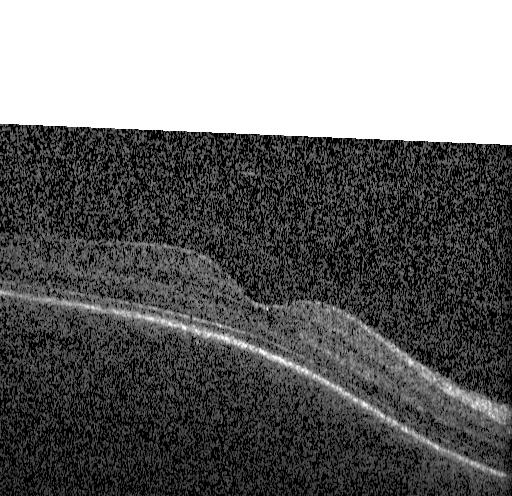

SD-OCT; retinal OCT B-scan; through the macula; instrument: Heidelberg Spectralis
Finding: neither CNV, DME, nor drusen.